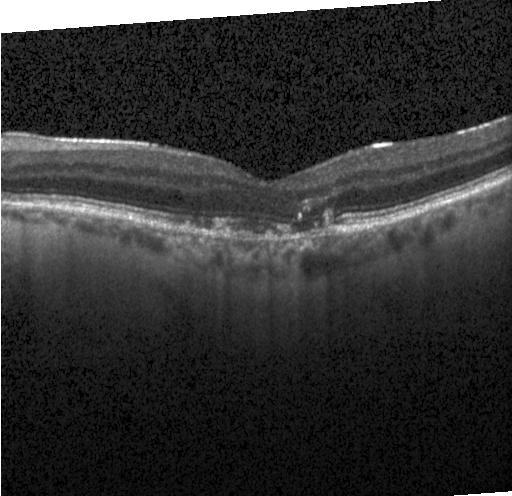 OCT scan showing a choroidal neovascular membrane.